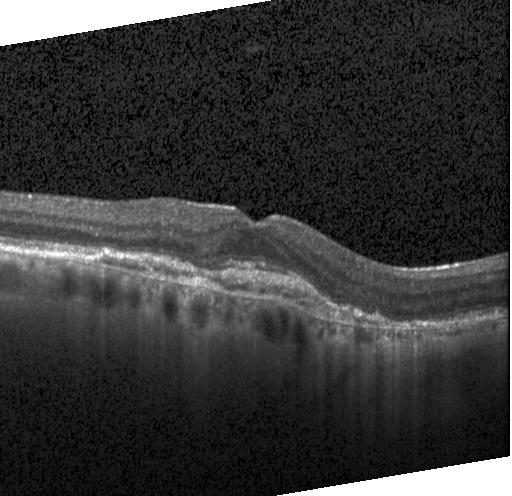 Assessment: choroidal neovascularization.